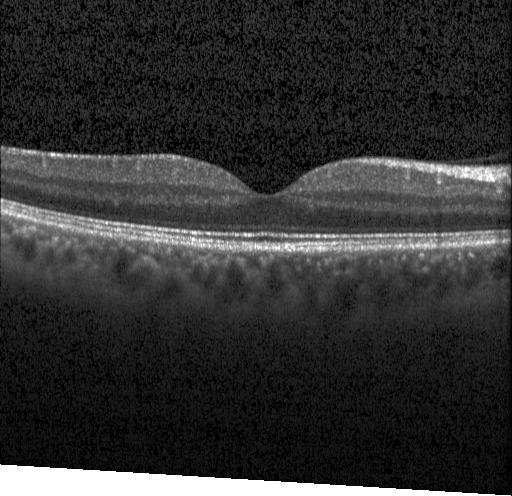 The scan shows no choroidal neovascularization, no diabetic macular edema, and no drusen.